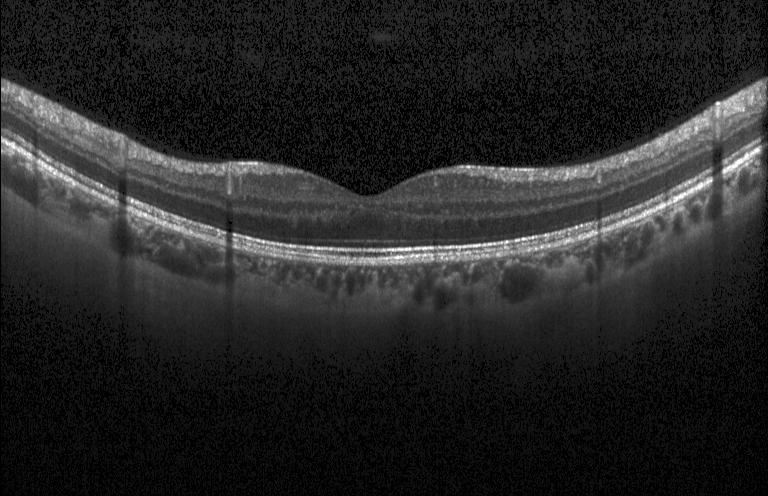

OCT B-scan
Finding: no choroidal neovascularization, diabetic macular edema, or drusen.